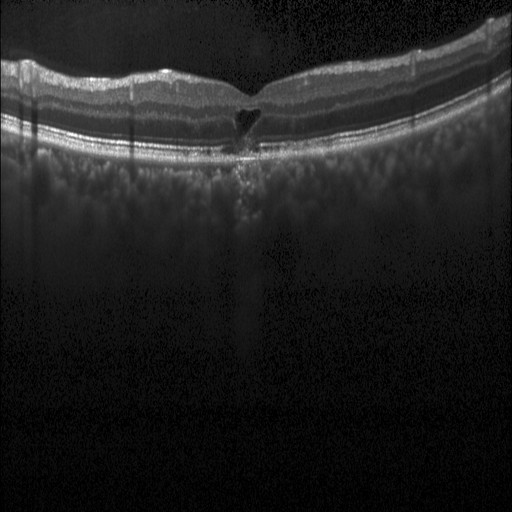
Impression: DME.